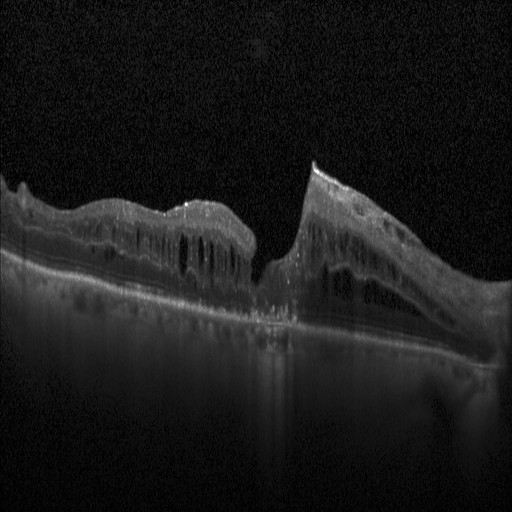

Optical coherence tomography scan, SD-OCT. Dx: diabetic macular edema (DME).